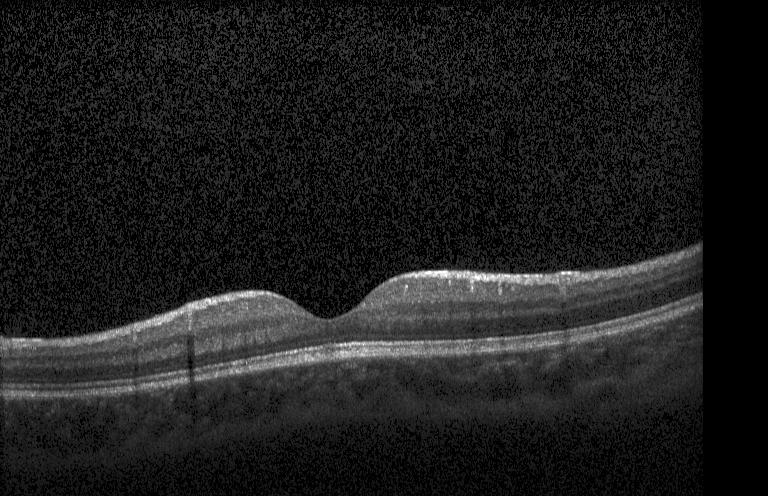 OCT B-scan, instrument: Heidelberg Spectralis, spectral-domain OCT. Neither choroidal neovascularization, diabetic macular edema, nor drusen.